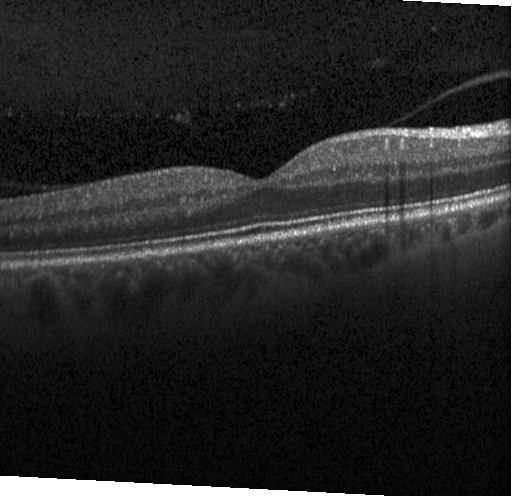
Fovea-centered; acquired on a Heidelberg Spectralis; OCT line scan — Macular OCT: neither choroidal neovascularization, diabetic macular edema, nor drusen.